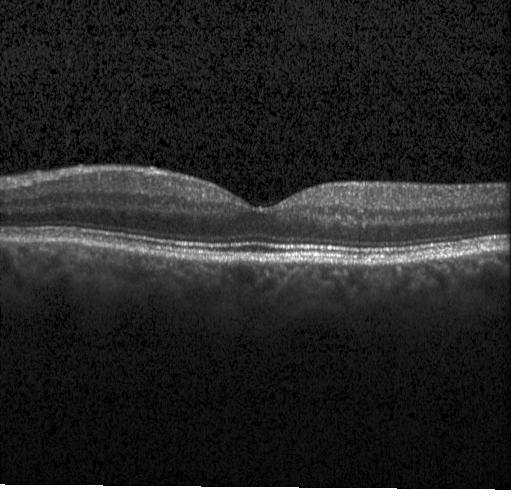 Retinal OCT B-scan. No choroidal neovascularization, diabetic macular edema, or drusen.